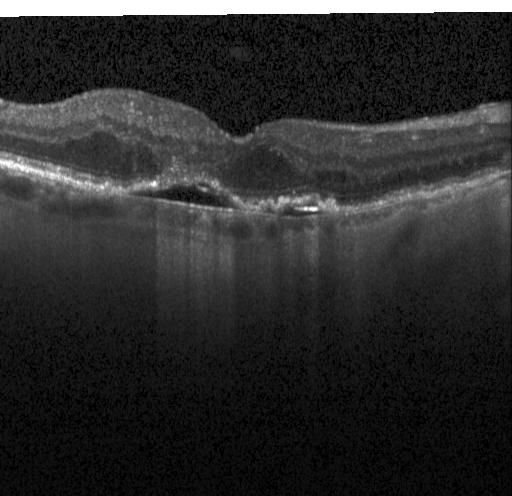 Horizontal scan through the fovea. Heidelberg Spectralis OCT system. Spectral-domain optical coherence tomography. Retinal OCT cross-section. OCT finding: a choroidal neovascular membrane.